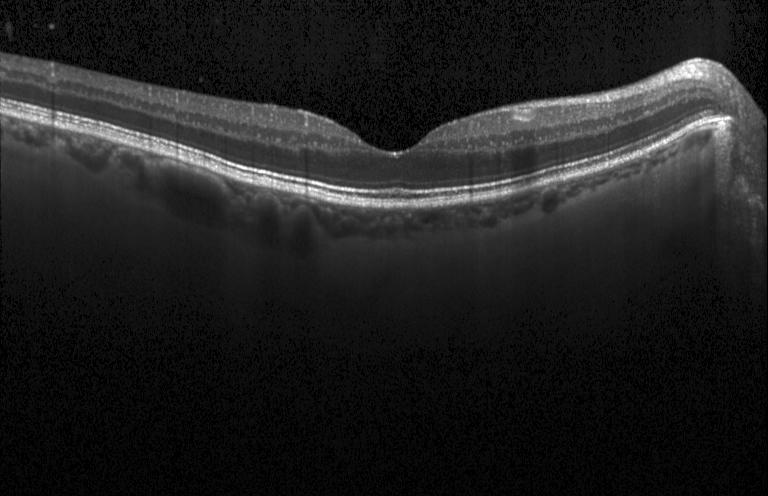

OCT line scan
Assessment: no choroidal neovascularization, diabetic macular edema, or drusen.